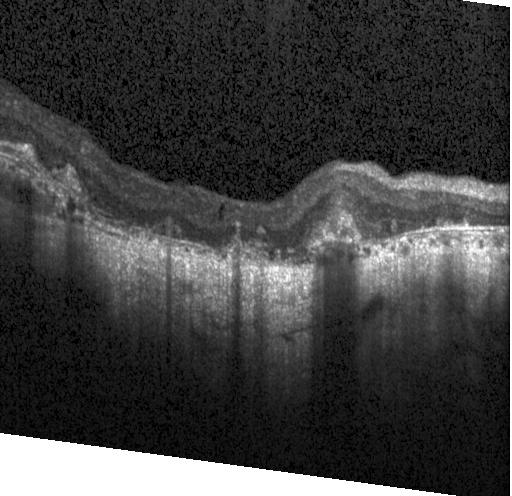 OCT B-scan. Acquired on a Heidelberg Spectralis. Spectral-domain optical coherence tomography. Diagnosis: choroidal neovascularization.